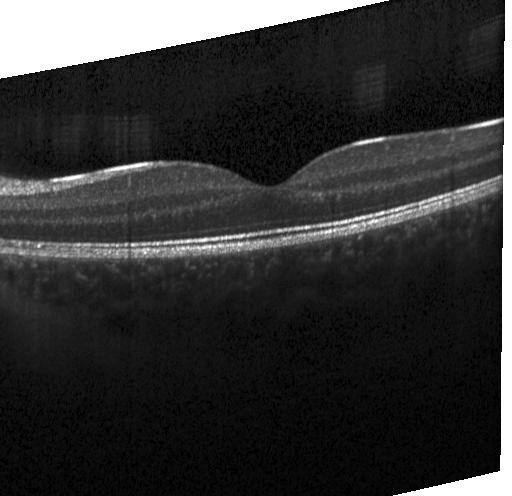 Dx: no evidence of choroidal neovascularization, diabetic macular edema, or drusen.